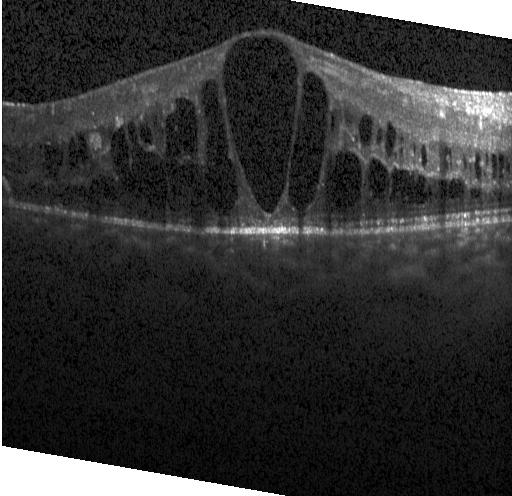
Spectral-domain OCT · optical coherence tomography scan · acquired on a Heidelberg Spectralis. Impression: diabetic macular edema.